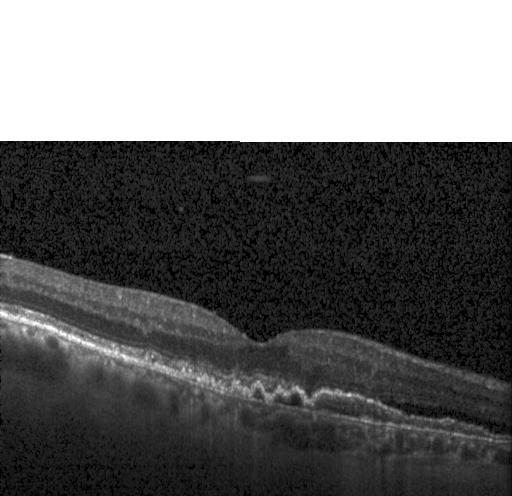 OCT B-scan. Macular OCT: a choroidal neovascular membrane.